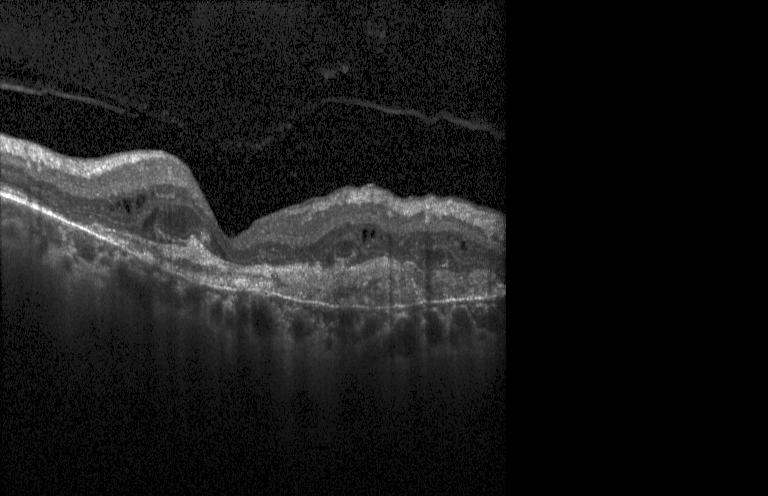
Optical coherence tomography B-scan.
Diagnosis: a choroidal neovascular membrane.